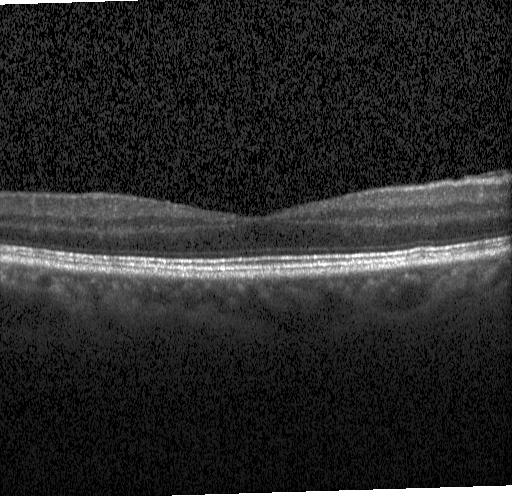

Optical coherence tomography B-scan
Macular OCT: neither choroidal neovascularization, diabetic macular edema, nor drusen.